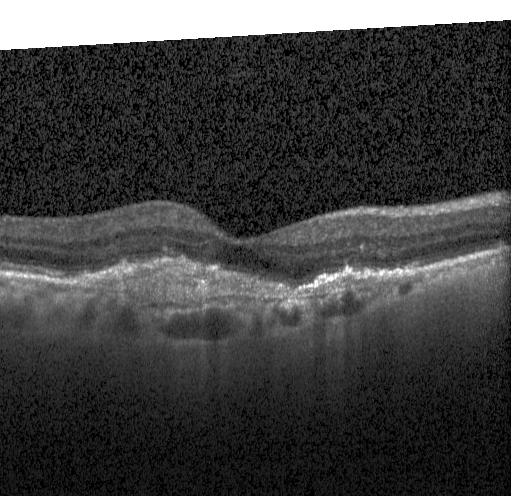
Retinal OCT cross-section. Heidelberg Spectralis.
Impression: a choroidal neovascular membrane.